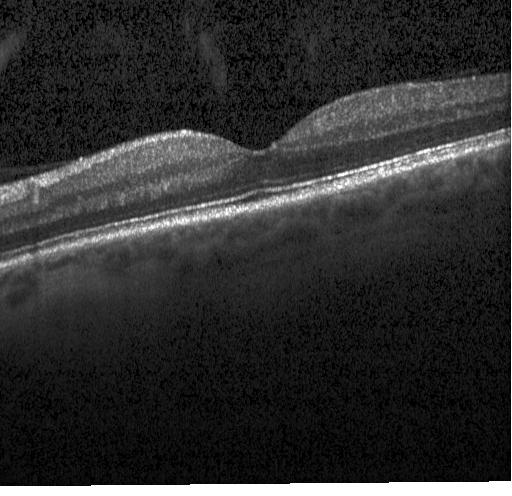
Heidelberg Spectralis, OCT line scan
Diagnosis: neither CNV, DME, nor drusen.